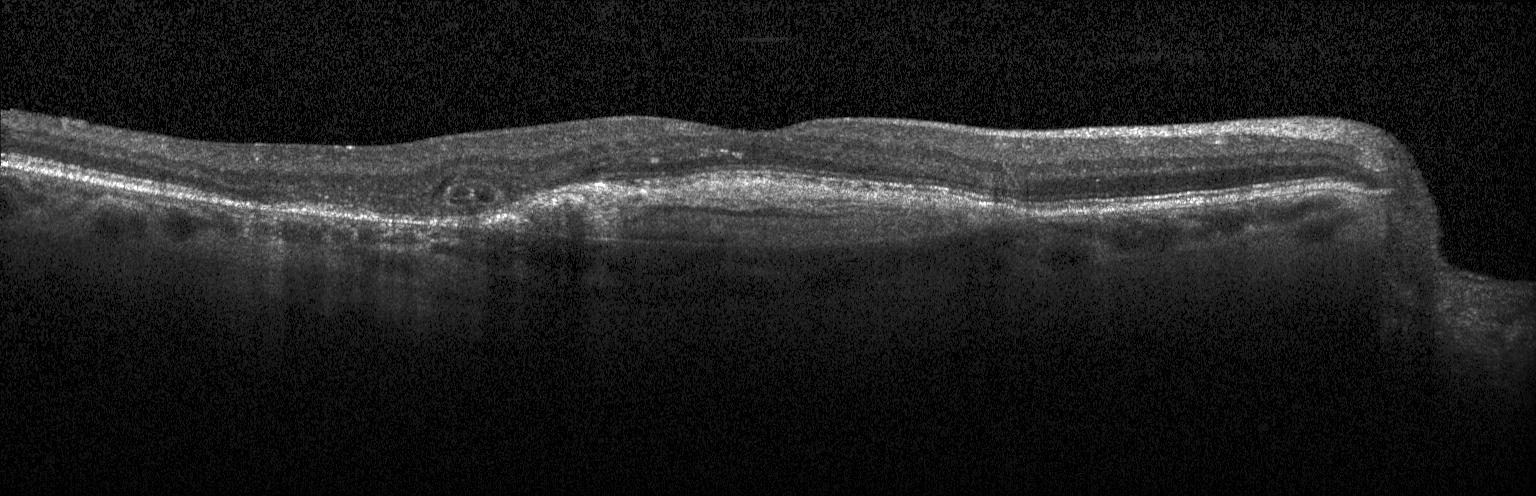 Optical coherence tomography scan.
Dx: a choroidal neovascular membrane.